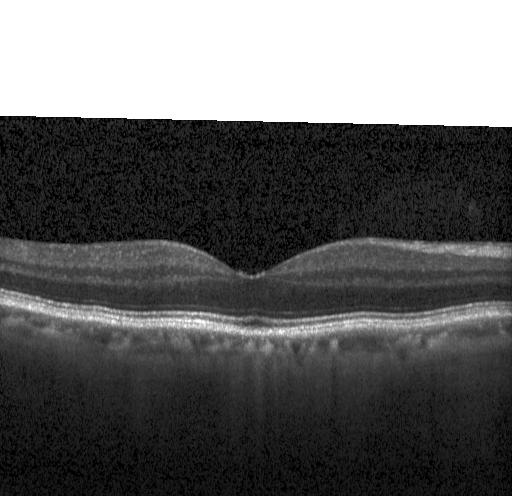

Centered on the fovea. Spectral-domain optical coherence tomography. Retinal OCT B-scan — Impression: no choroidal neovascularization, diabetic macular edema, or drusen.